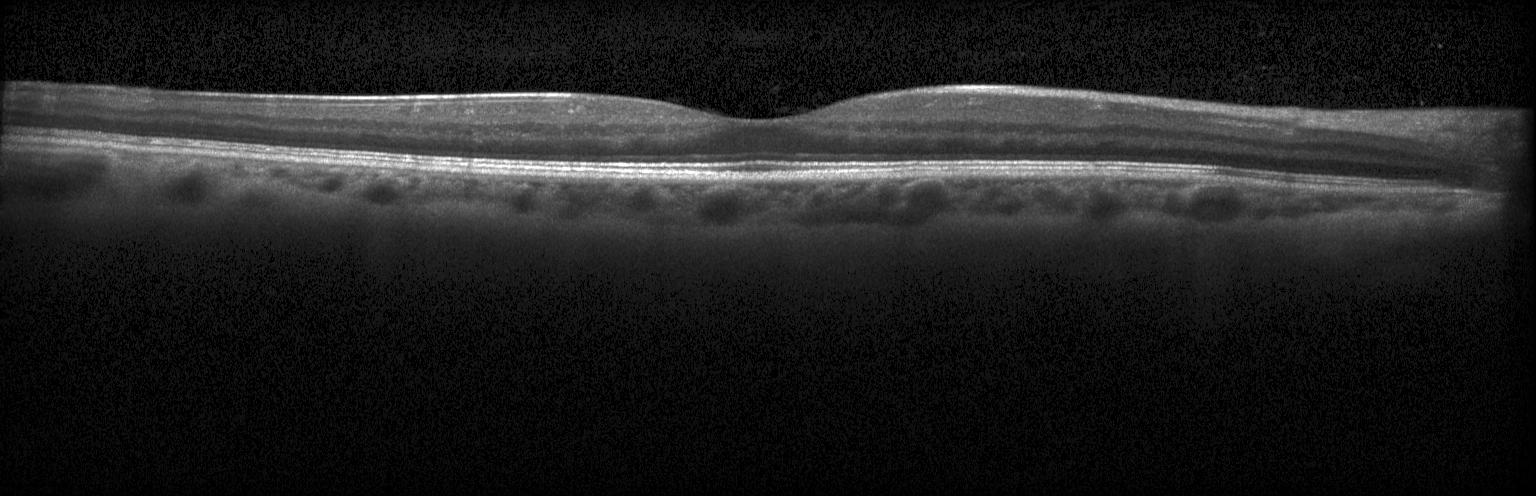
OCT finding: no choroidal neovascularization, no diabetic macular edema, and no drusen.